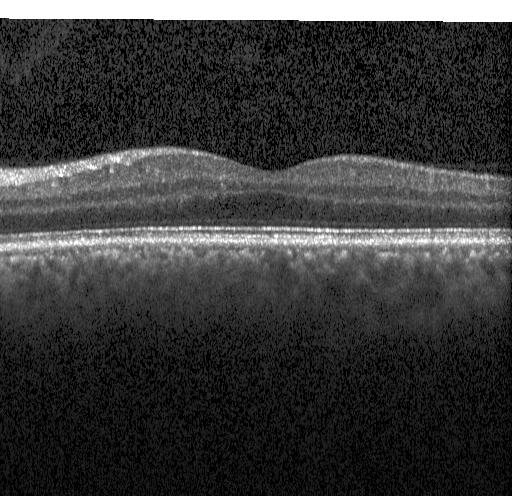
OCT B-scan · acquired on a Heidelberg Spectralis · horizontal scan through the fovea · spectral-domain optical coherence tomography — Assessment: neither choroidal neovascularization, diabetic macular edema, nor drusen.